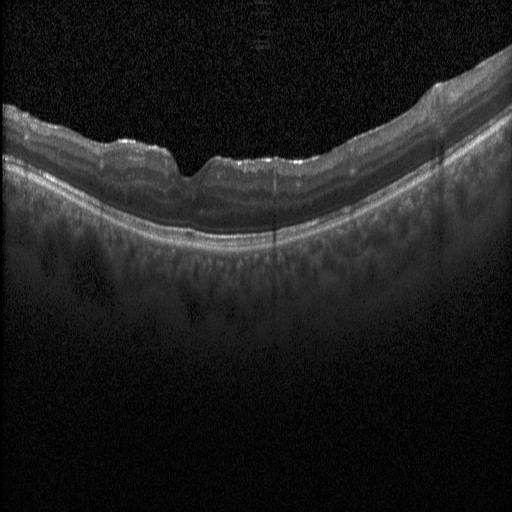

Through the macula; OCT B-scan
The scan shows diabetic macular edema.